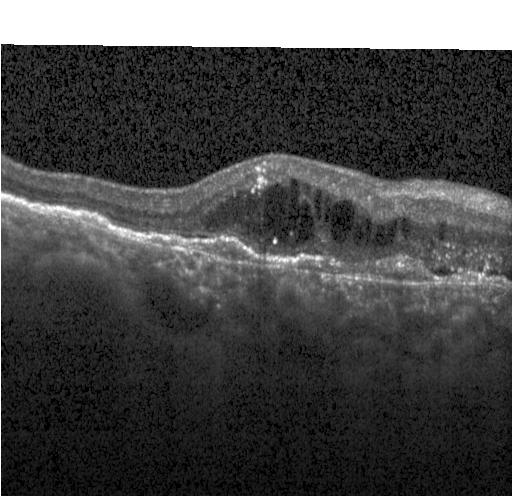 Diagnosis: choroidal neovascularization.